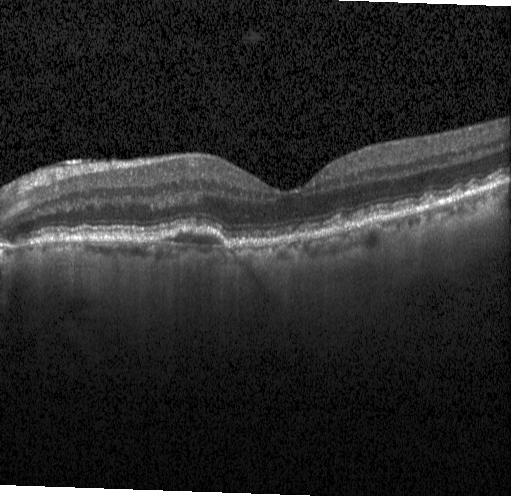

OCT finding: a choroidal neovascular membrane.